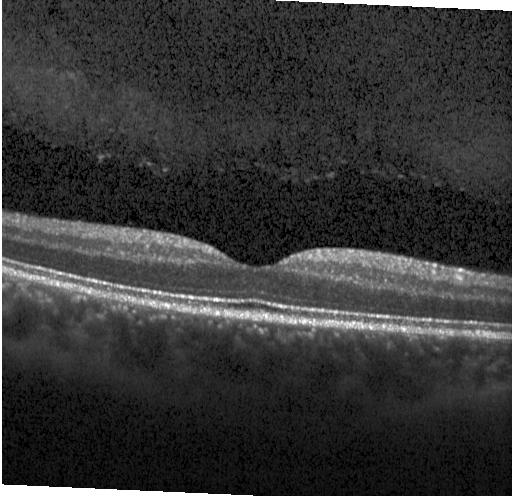

Macular scan, SD-OCT, optical coherence tomography scan, Heidelberg Spectralis. Impression: no evidence of CNV, DME, or drusen.